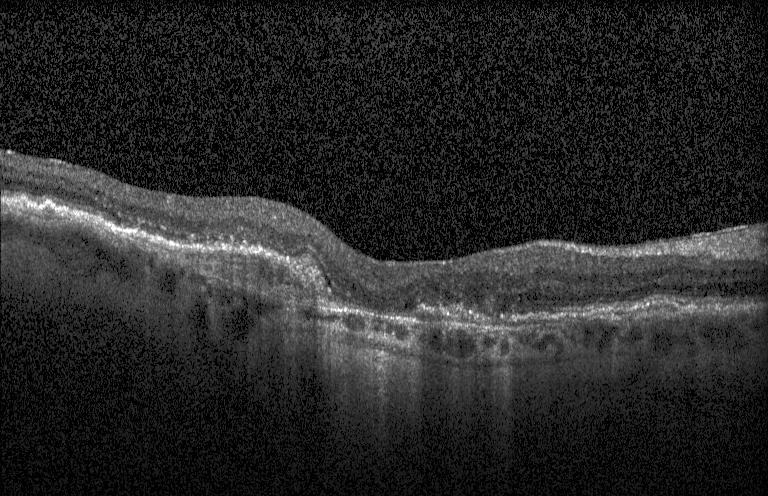

Horizontal scan through the fovea, SD-OCT, optical coherence tomography scan, Heidelberg Spectralis
Macular OCT: a choroidal neovascular membrane.